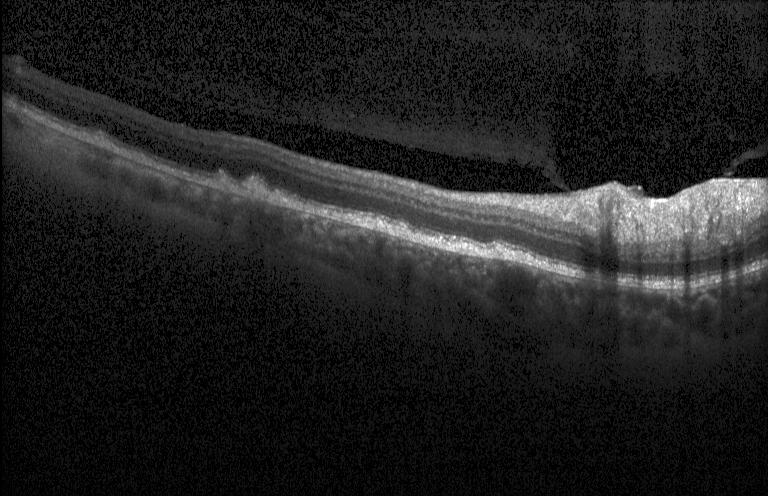 Optical coherence tomography scan. Horizontal scan through the fovea. Diagnosis: multiple drusen.